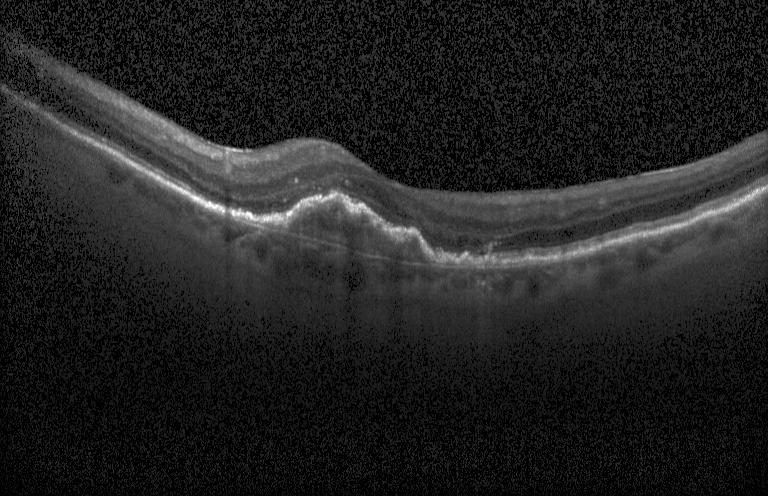

Optical coherence tomography B-scan · fovea-centered · spectral-domain optical coherence tomography. OCT finding: a choroidal neovascular membrane.